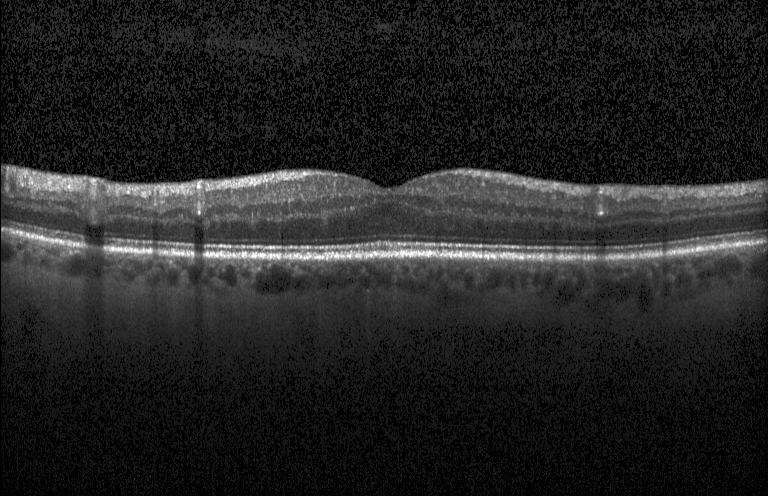
OCT line scan
Diagnosis: neither choroidal neovascularization, diabetic macular edema, nor drusen.